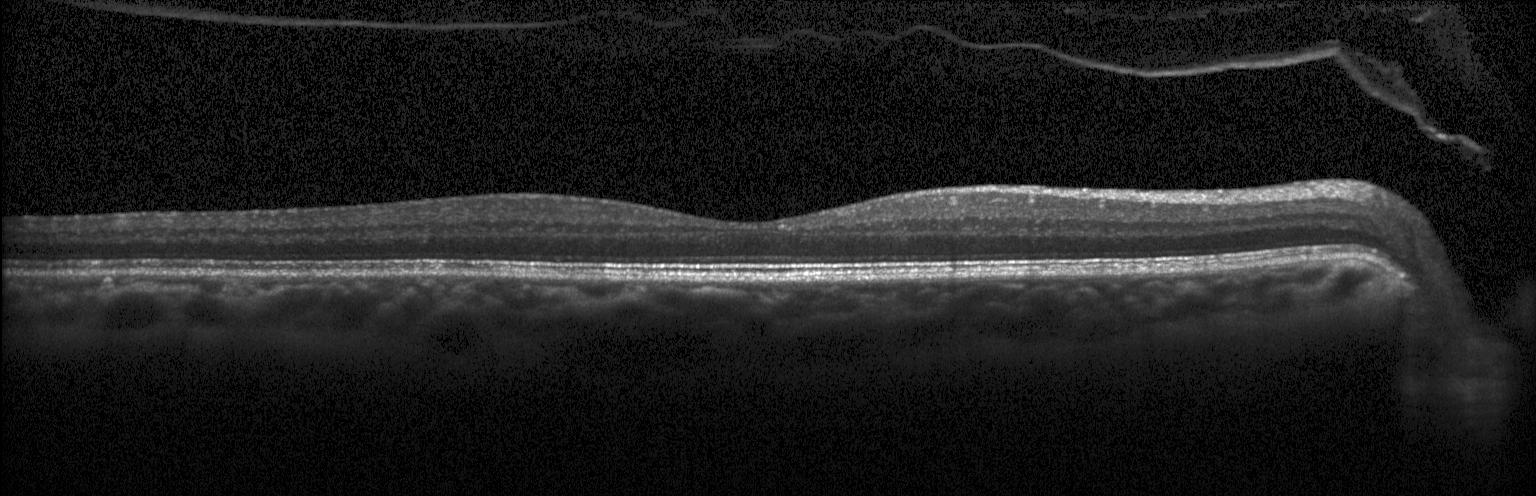

Optical coherence tomography scan; Heidelberg Spectralis OCT system; spectral-domain optical coherence tomography; through the macula — Dx: no CNV, no DME, and no drusen.